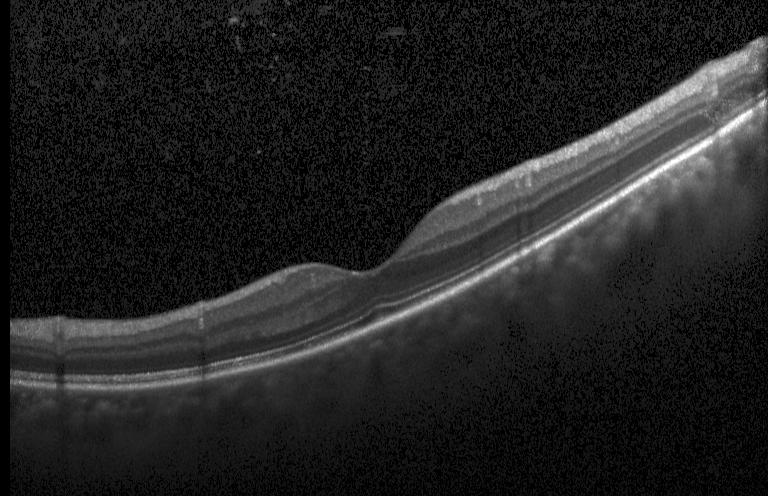 Spectral-domain optical coherence tomography, fovea-centered, acquired on a Heidelberg Spectralis, optical coherence tomography scan
This B-scan demonstrates no evidence of choroidal neovascularization, diabetic macular edema, or drusen.